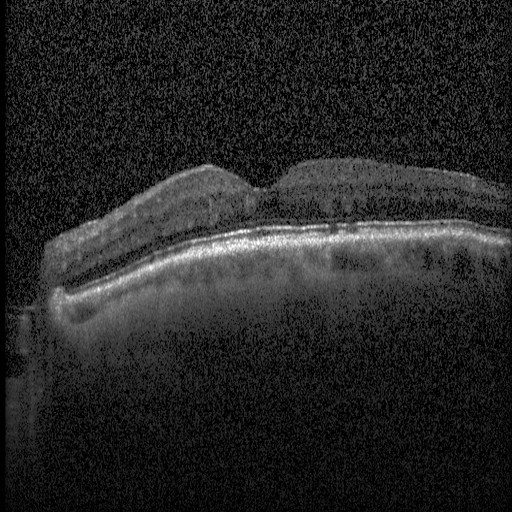 Retinal OCT B-scan, fovea-centered
Diagnosis: DME.